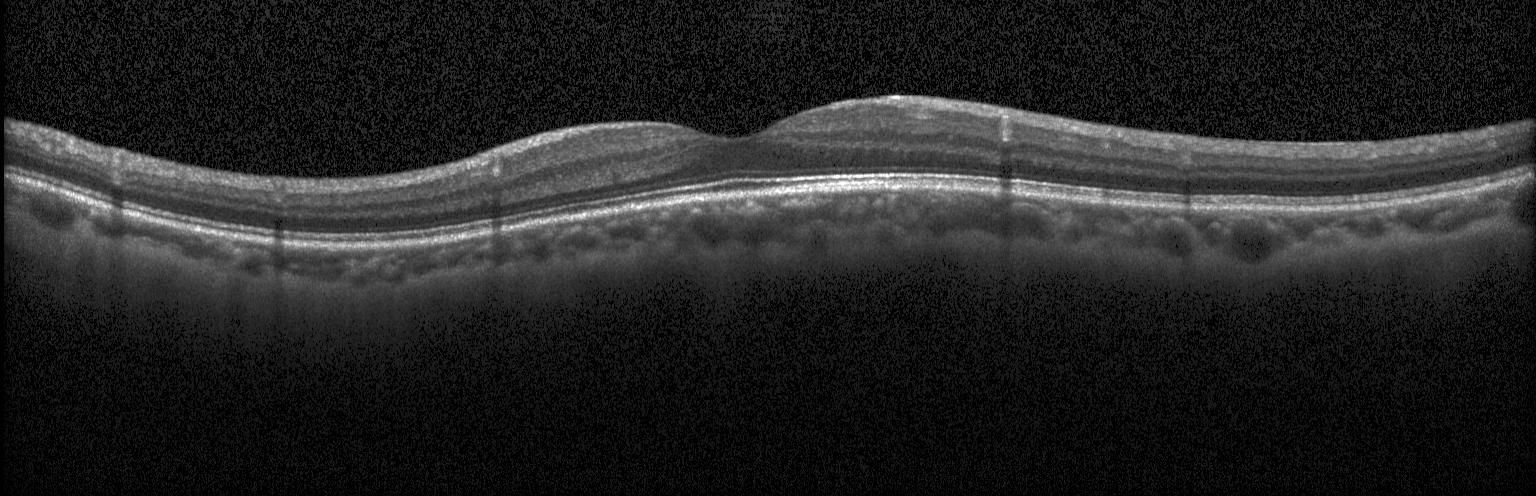
Retinal OCT B-scan; spectral-domain optical coherence tomography — Finding: no choroidal neovascularization, no diabetic macular edema, and no drusen.